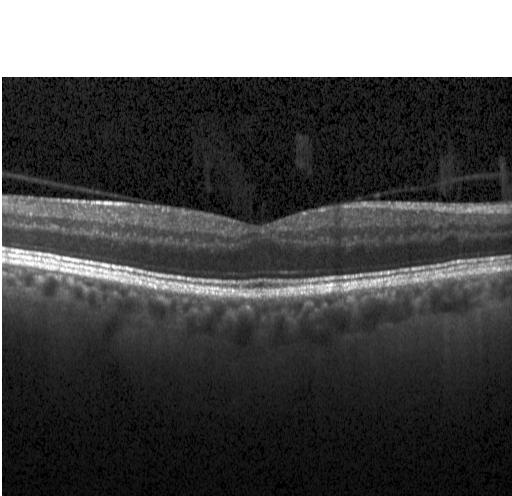

Retinal OCT cross-section, instrument: Heidelberg Spectralis. Diagnosis: no choroidal neovascularization, diabetic macular edema, or drusen.